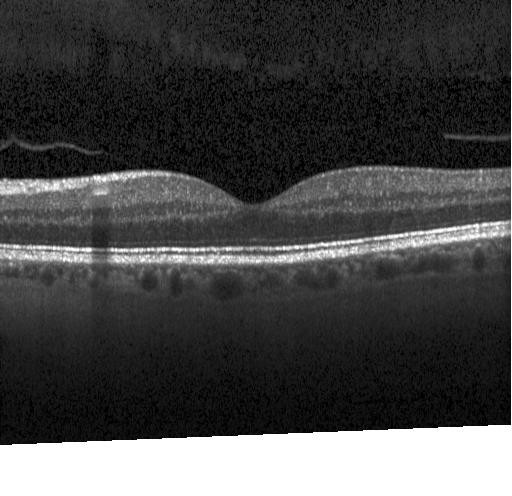 Retinal OCT B-scan — Impression: no choroidal neovascularization, diabetic macular edema, or drusen.